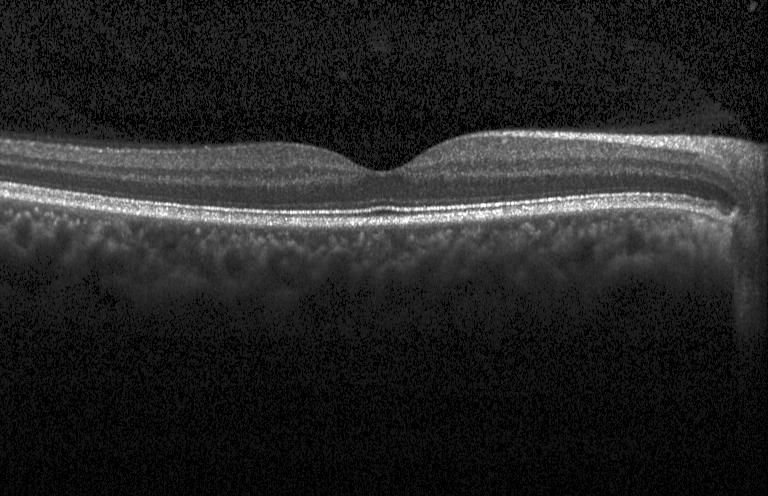
Retinal OCT cross-section · spectral-domain OCT — Finding: no choroidal neovascularization, diabetic macular edema, or drusen.